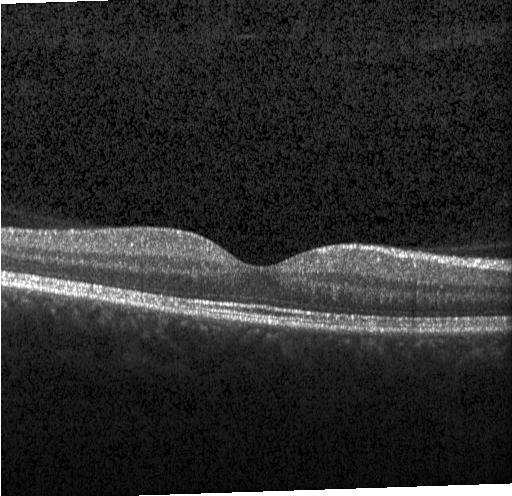
OCT B-scan · centered on the fovea — The scan shows neither choroidal neovascularization, diabetic macular edema, nor drusen.